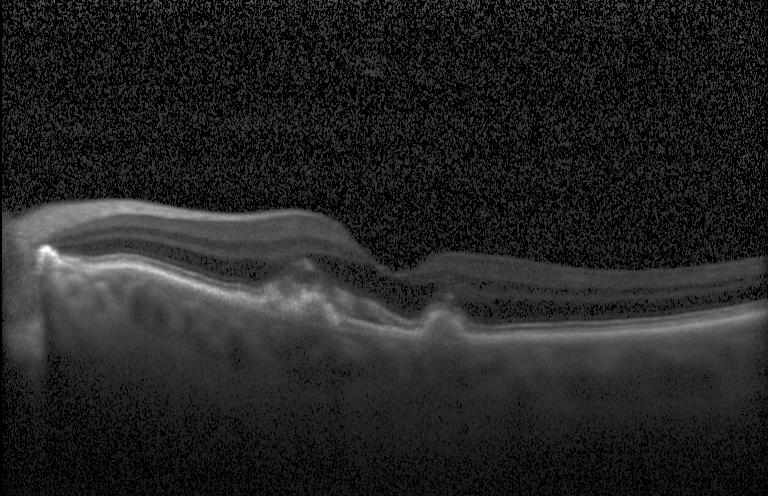 OCT B-scan — Diagnosis: a choroidal neovascular membrane.